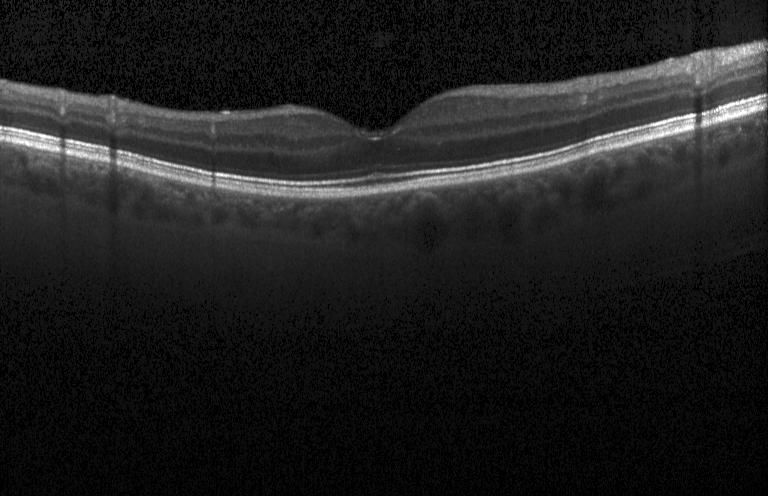

OCT finding: no choroidal neovascularization, diabetic macular edema, or drusen.